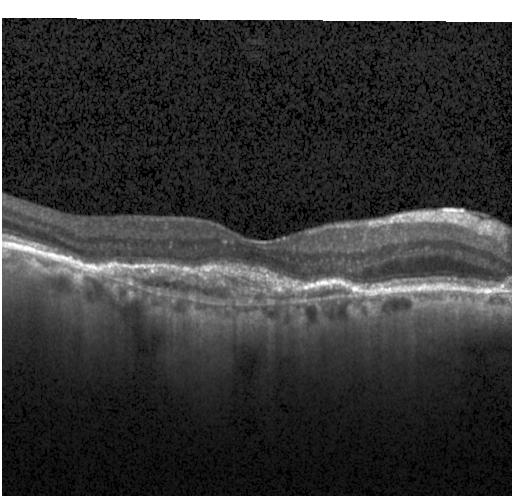 Optical coherence tomography B-scan
Diagnosis: CNV.